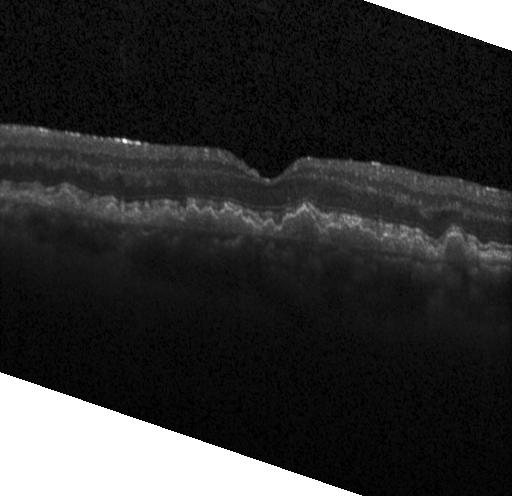

Spectral-domain OCT B-scan: choroidal neovascularization (CNV).